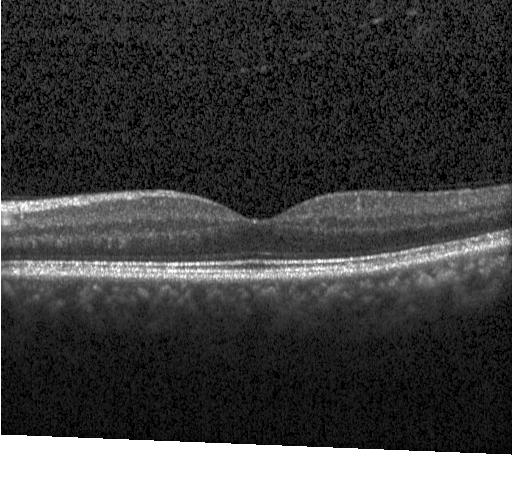

Diagnosis: neither choroidal neovascularization, diabetic macular edema, nor drusen.